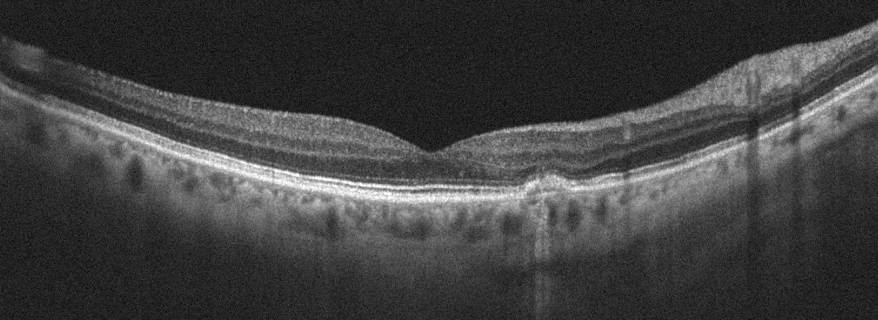
Impression: AMD.